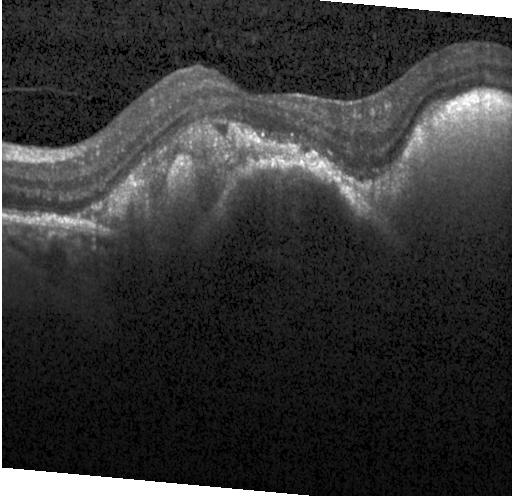

Choroidal neovascularization (CNV).